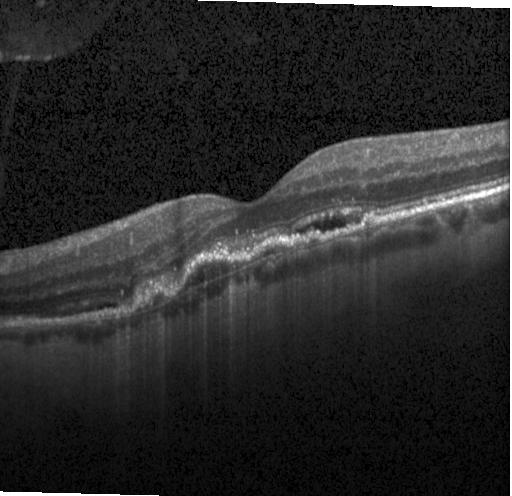 Centered on the fovea, retinal OCT cross-section — Diagnosis: a choroidal neovascular membrane.